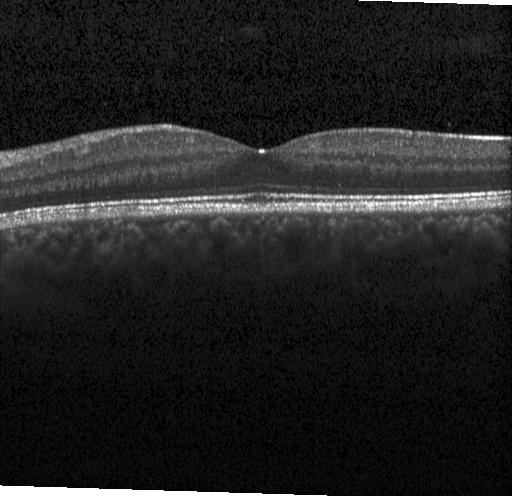
Centered on the fovea · spectral-domain OCT · acquired on a Heidelberg Spectralis · OCT line scan
Macular OCT: no choroidal neovascularization, diabetic macular edema, or drusen.